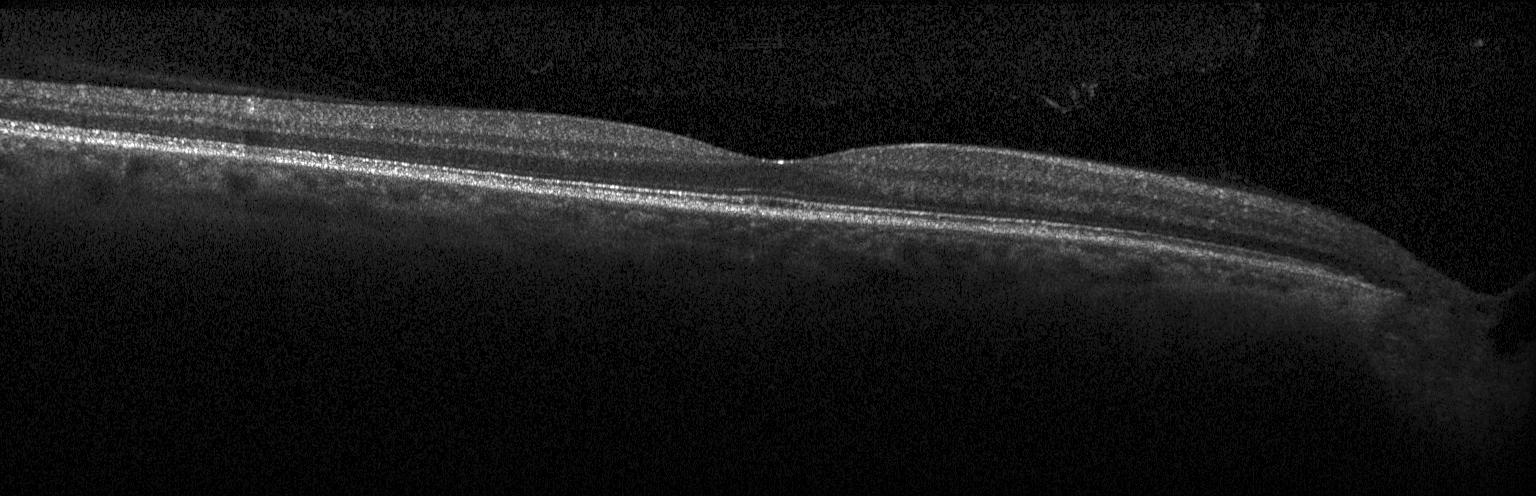
Fovea-centered. Optical coherence tomography B-scan. Spectral-domain optical coherence tomography. Acquired on a Heidelberg Spectralis.
Finding: neither choroidal neovascularization, diabetic macular edema, nor drusen.